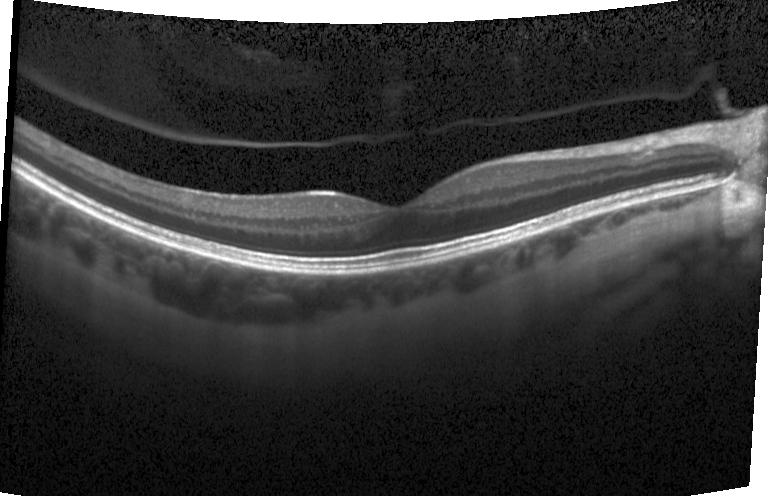
Impression: no CNV, no DME, and no drusen.